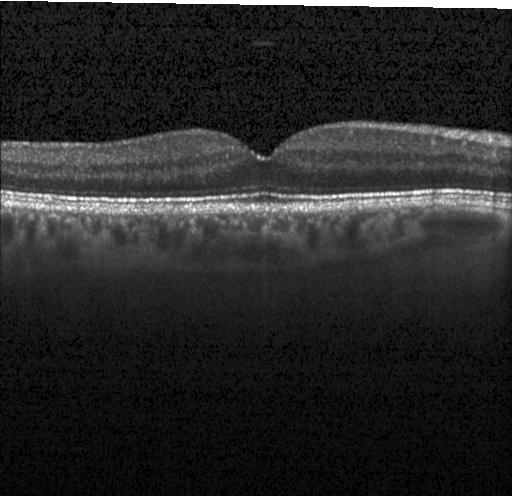

Diagnosis: no choroidal neovascularization, diabetic macular edema, or drusen.